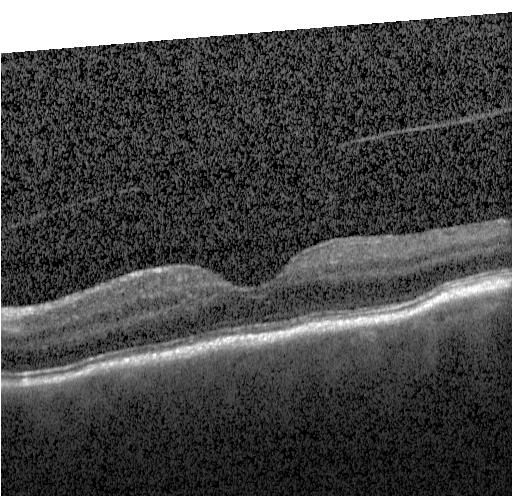

Spectral-domain OCT; Heidelberg Spectralis OCT system; OCT B-scan; centered on the fovea — Diagnosis: no evidence of choroidal neovascularization, diabetic macular edema, or drusen.